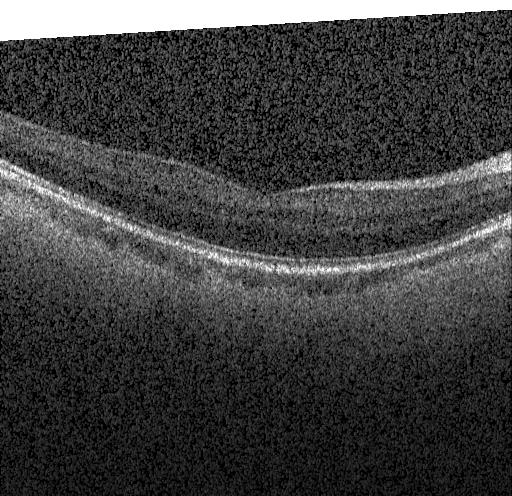 The scan shows no evidence of choroidal neovascularization, diabetic macular edema, or drusen.